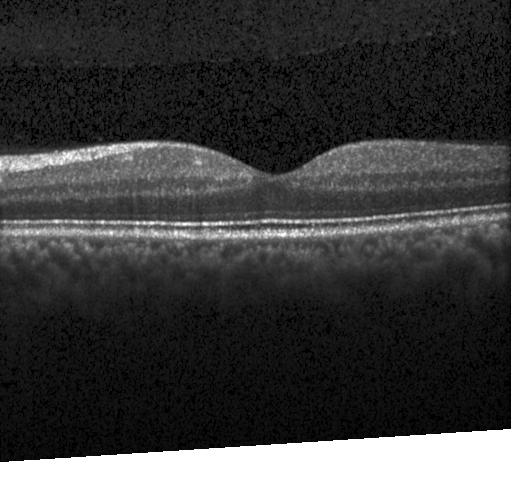
Optical coherence tomography B-scan. Instrument: Heidelberg Spectralis. OCT finding: no evidence of CNV, DME, or drusen.